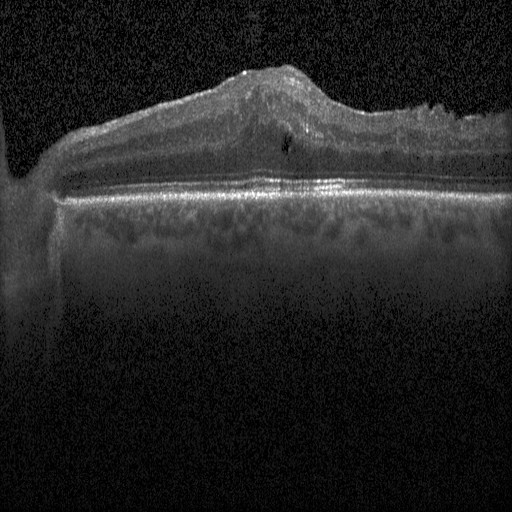
Retinal OCT cross-section — The scan shows DME.